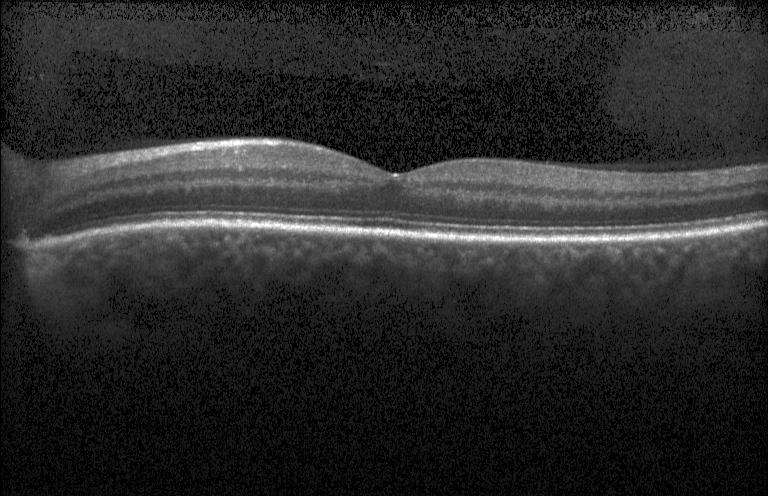
Spectral-domain OCT B-scan: no CNV, DME, or drusen.